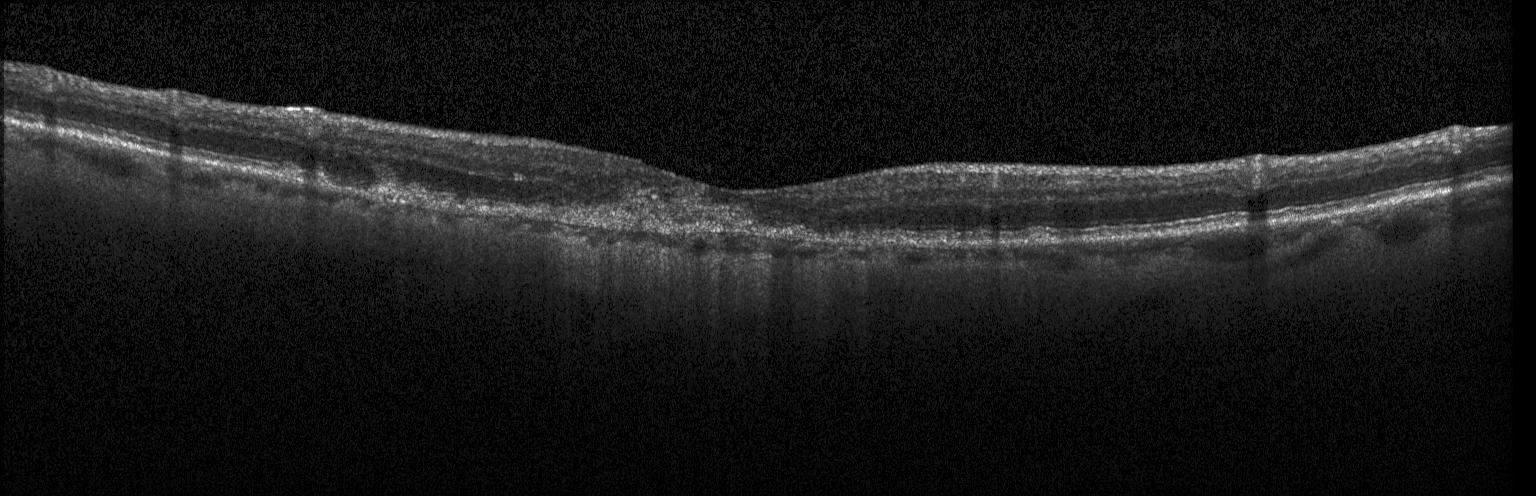 OCT line scan; instrument: Heidelberg Spectralis — OCT finding: a choroidal neovascular membrane.